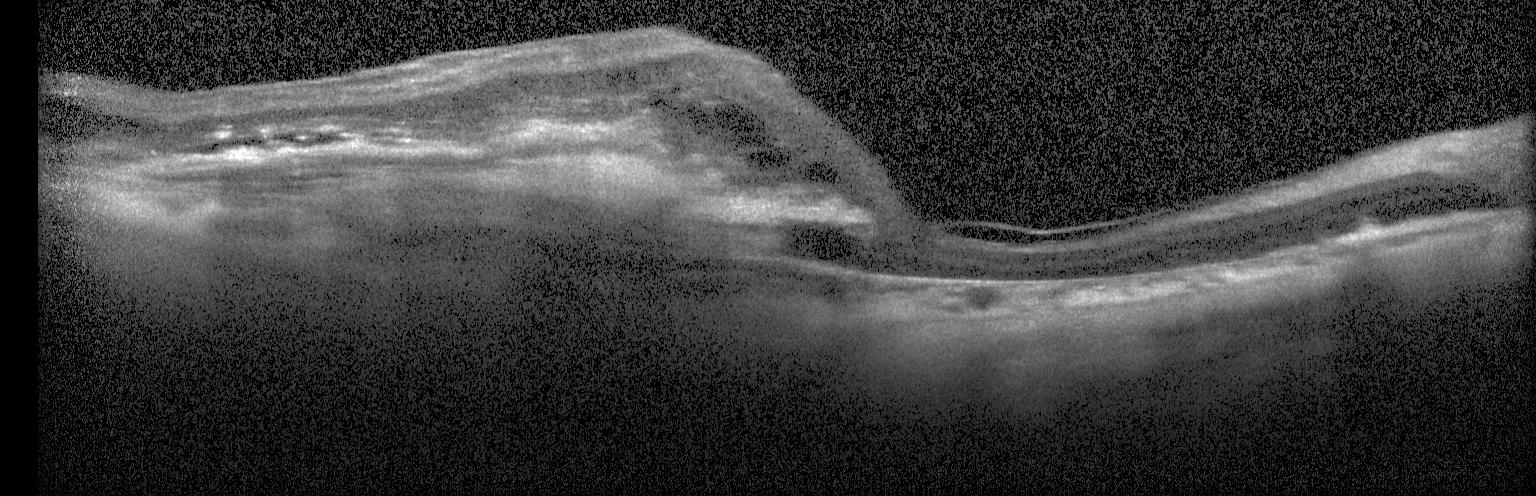 OCT B-scan · SD-OCT
The scan shows a choroidal neovascular membrane.